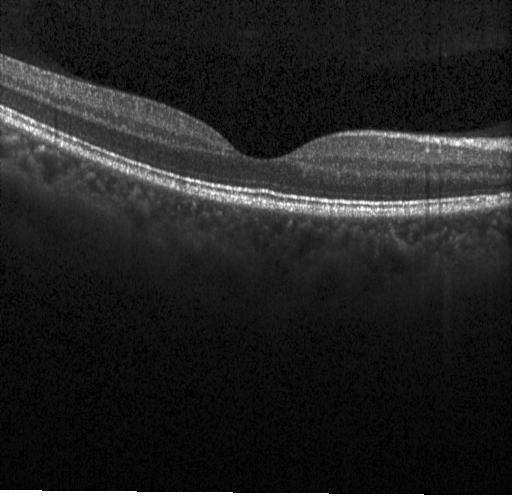

Macular OCT: no choroidal neovascularization, diabetic macular edema, or drusen.